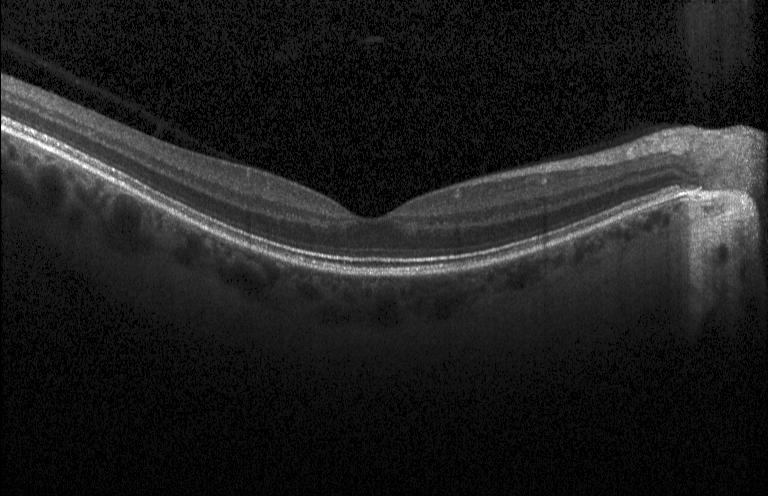

SD-OCT; retinal OCT B-scan; horizontal scan through the fovea.
No CNV, DME, or drusen.